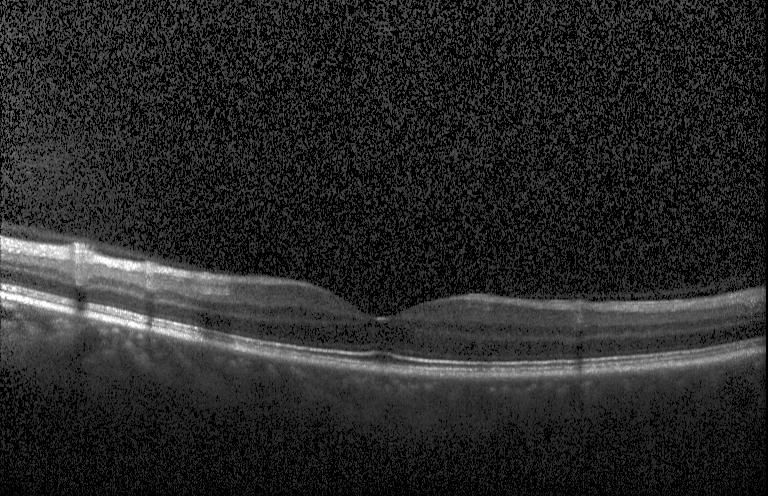 Acquired on a Heidelberg Spectralis. Retinal OCT cross-section. Spectral-domain optical coherence tomography. No CNV, no DME, and no drusen.